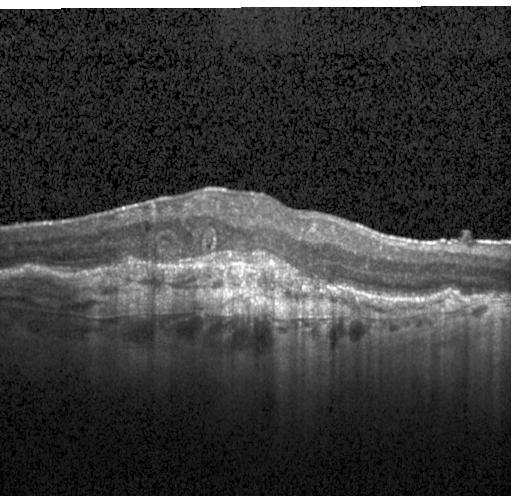
Retinal OCT B-scan; macular scan; SD-OCT; instrument: Heidelberg Spectralis
Assessment: CNV.